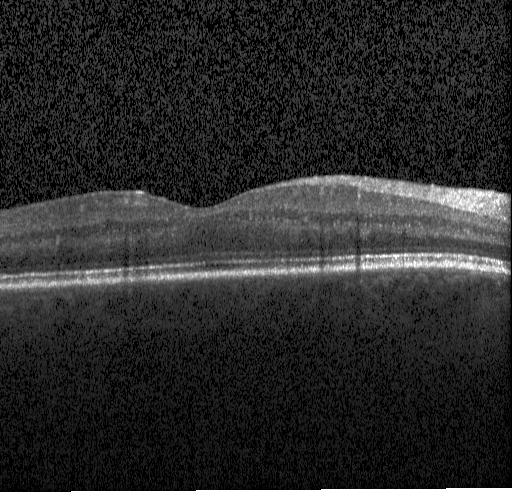
OCT line scan · spectral-domain optical coherence tomography · centered on the fovea · acquired on a Heidelberg Spectralis
Finding: no choroidal neovascularization, no diabetic macular edema, and no drusen.